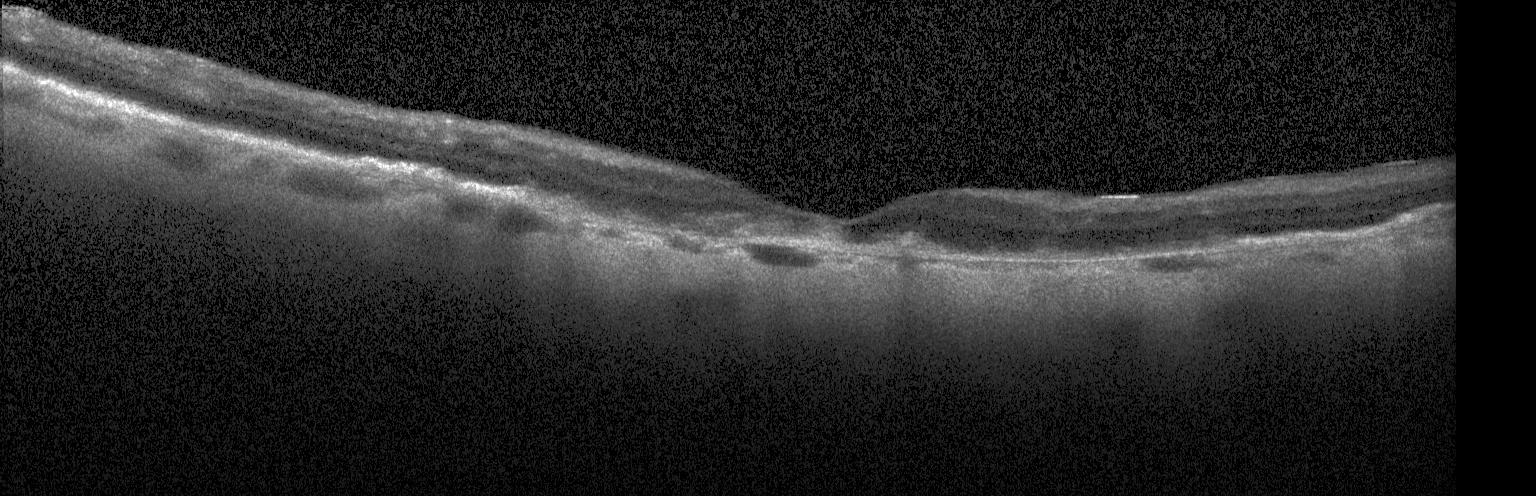

Spectral-domain OCT. Acquired on a Heidelberg Spectralis. Horizontal scan through the fovea. Retinal OCT cross-section
The scan shows CNV.